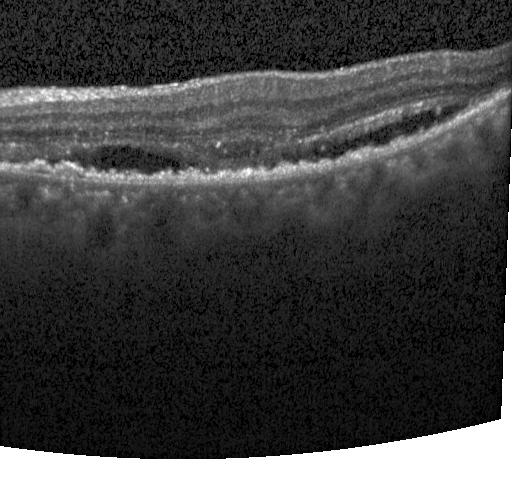
Optical coherence tomography scan. Diagnosis: CNV.